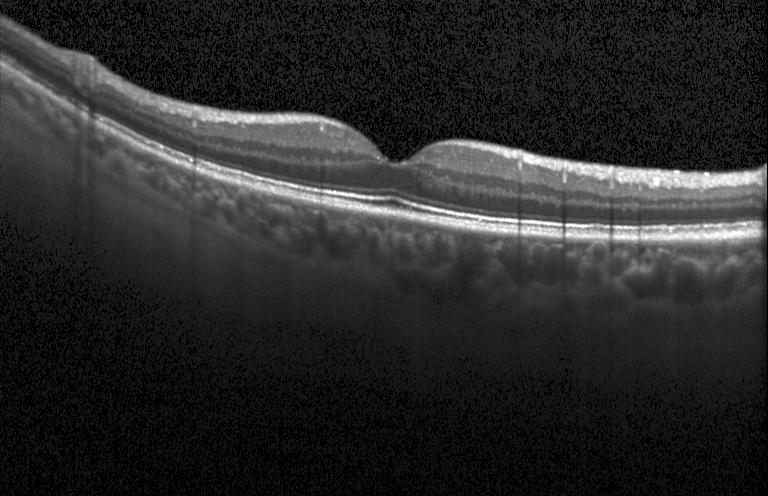

Heidelberg Spectralis OCT system. Through the macula. OCT line scan. This B-scan demonstrates neither choroidal neovascularization, diabetic macular edema, nor drusen.